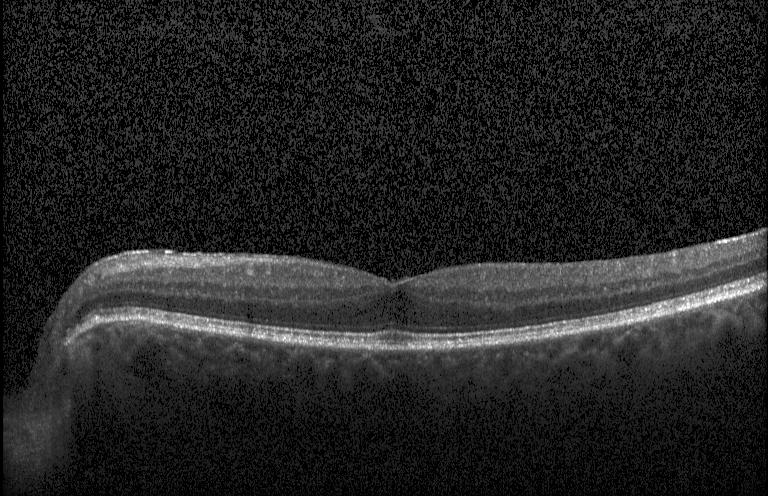

Optical coherence tomography scan, spectral-domain OCT.
Dx: no evidence of choroidal neovascularization, diabetic macular edema, or drusen.